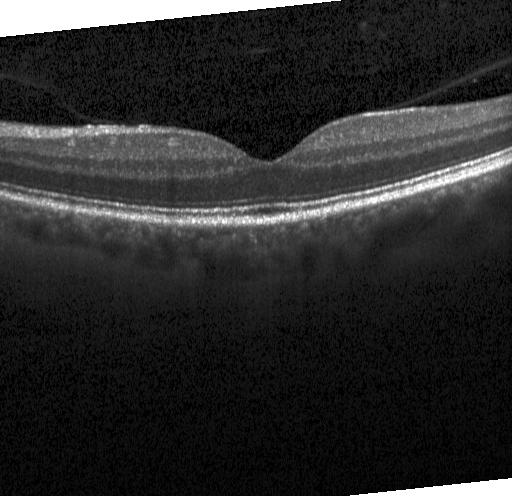

Dx: no evidence of choroidal neovascularization, diabetic macular edema, or drusen.